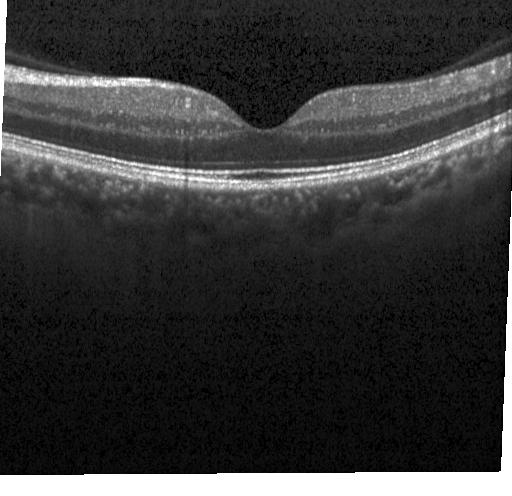
Fovea-centered. Heidelberg Spectralis. Optical coherence tomography scan. SD-OCT
Impression: neither choroidal neovascularization, diabetic macular edema, nor drusen.